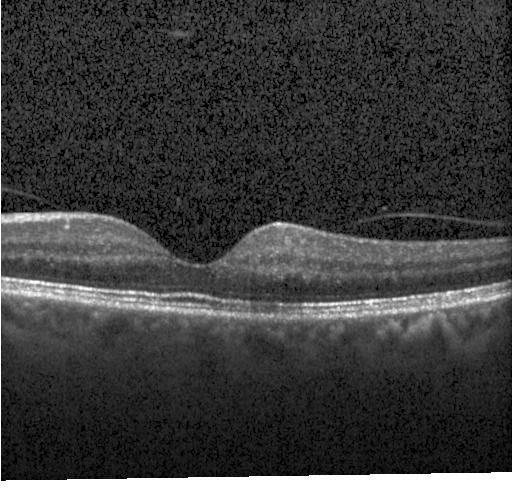
Spectral-domain OCT B-scan: no choroidal neovascularization, no diabetic macular edema, and no drusen.